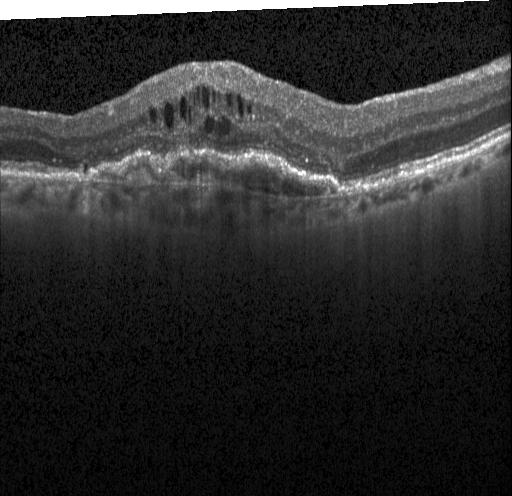

Macular OCT: a choroidal neovascular membrane.